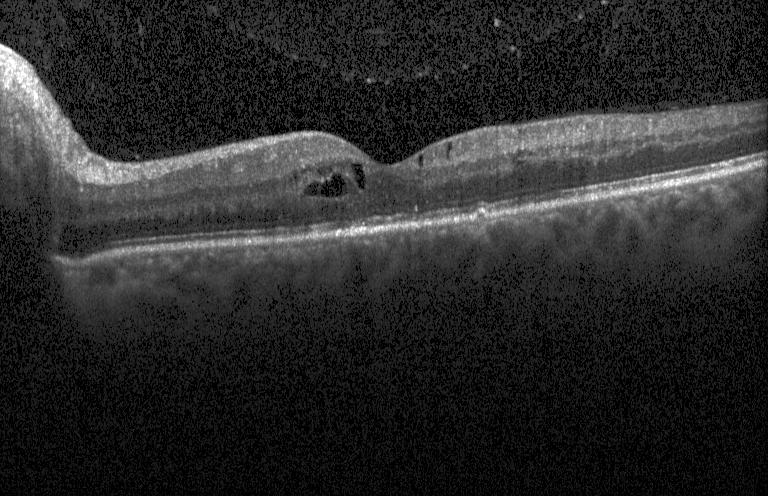
Retinal OCT B-scan.
The scan shows diabetic macular edema.